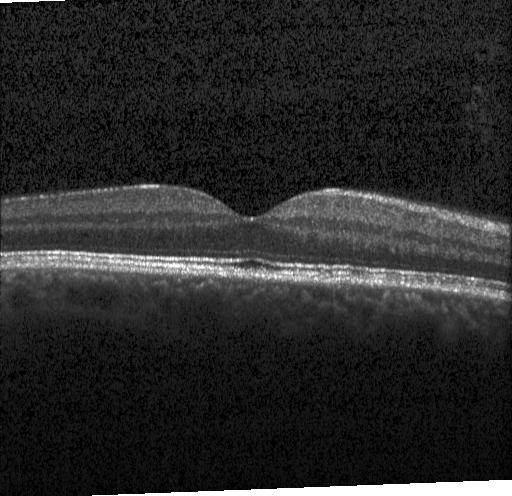

Spectral-domain optical coherence tomography; OCT B-scan; acquired on a Heidelberg Spectralis; centered on the fovea. Macular OCT: no evidence of choroidal neovascularization, diabetic macular edema, or drusen.